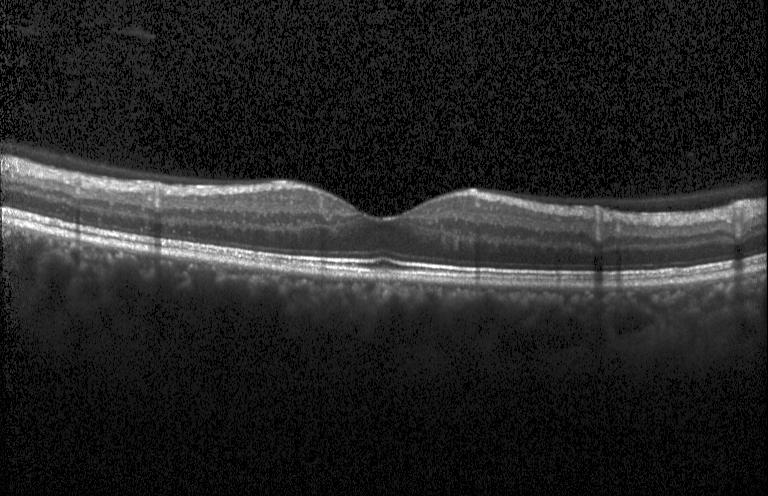

Retinal OCT B-scan.
OCT finding: no choroidal neovascularization, diabetic macular edema, or drusen.